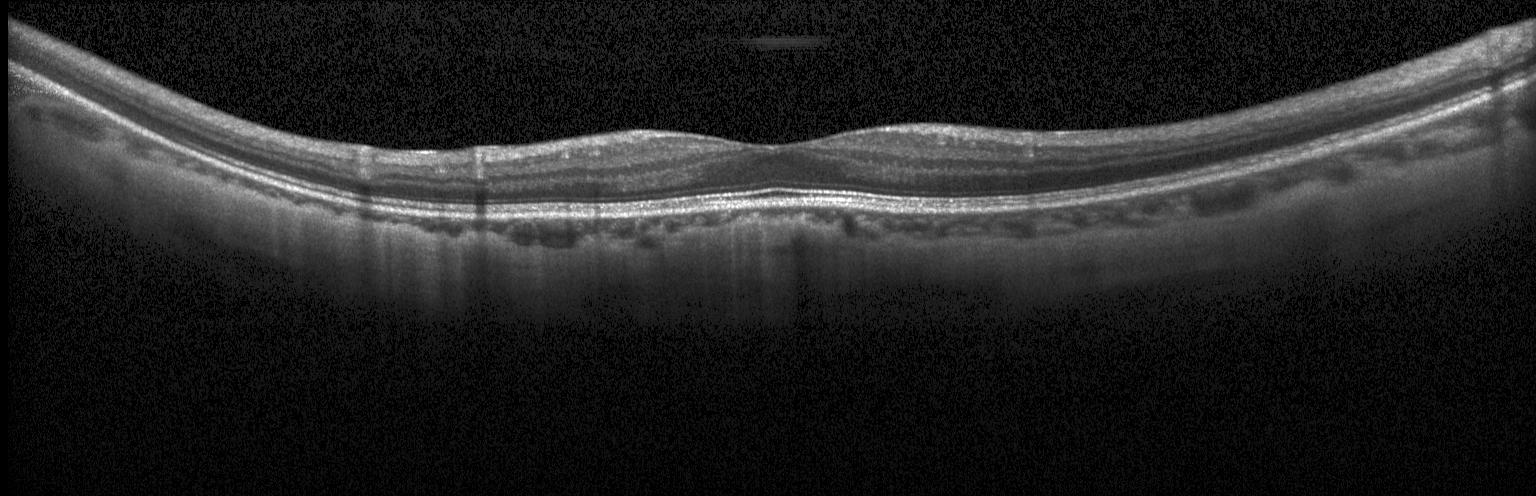

Dx: no choroidal neovascularization, no diabetic macular edema, and no drusen.